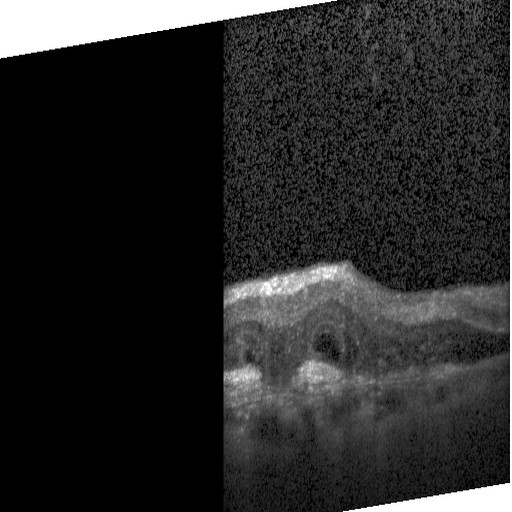 Retinal OCT cross-section. Assessment: DME.